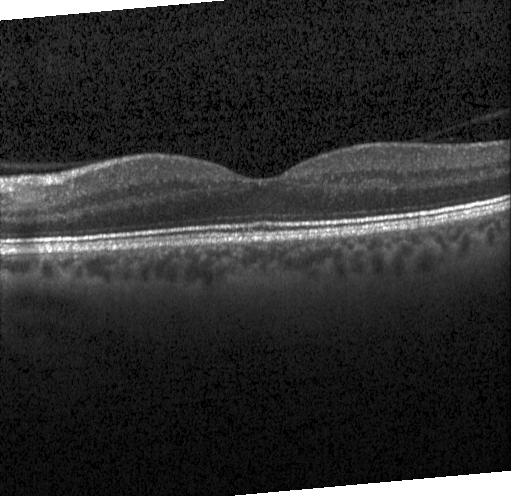
Macular OCT: no evidence of choroidal neovascularization, diabetic macular edema, or drusen.